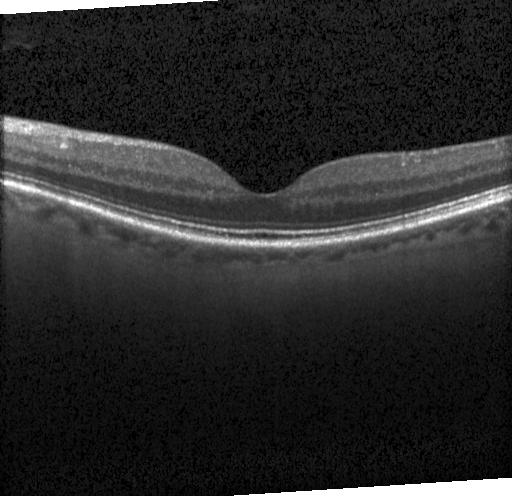

SD-OCT · macular scan · retinal OCT cross-section — Finding: no choroidal neovascularization, diabetic macular edema, or drusen.